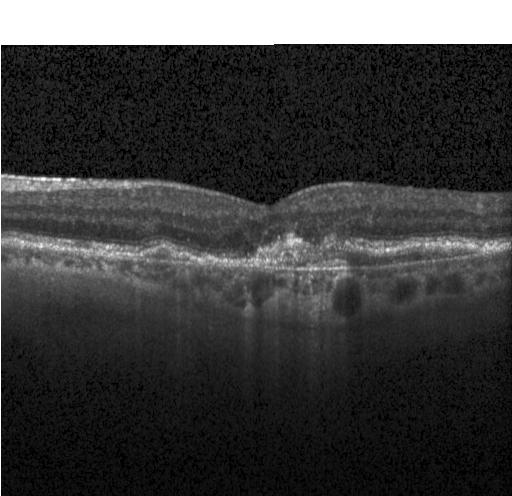 Spectral-domain optical coherence tomography. Heidelberg Spectralis. Through the macula. OCT B-scan. Macular OCT: CNV.